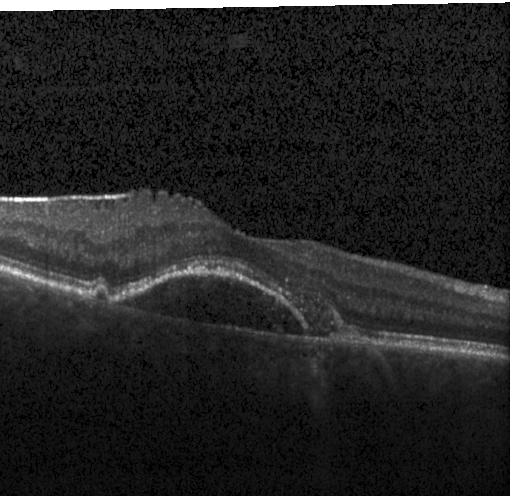

Spectral-domain OCT. Through the macula. Retinal OCT B-scan
OCT finding: a choroidal neovascular membrane.